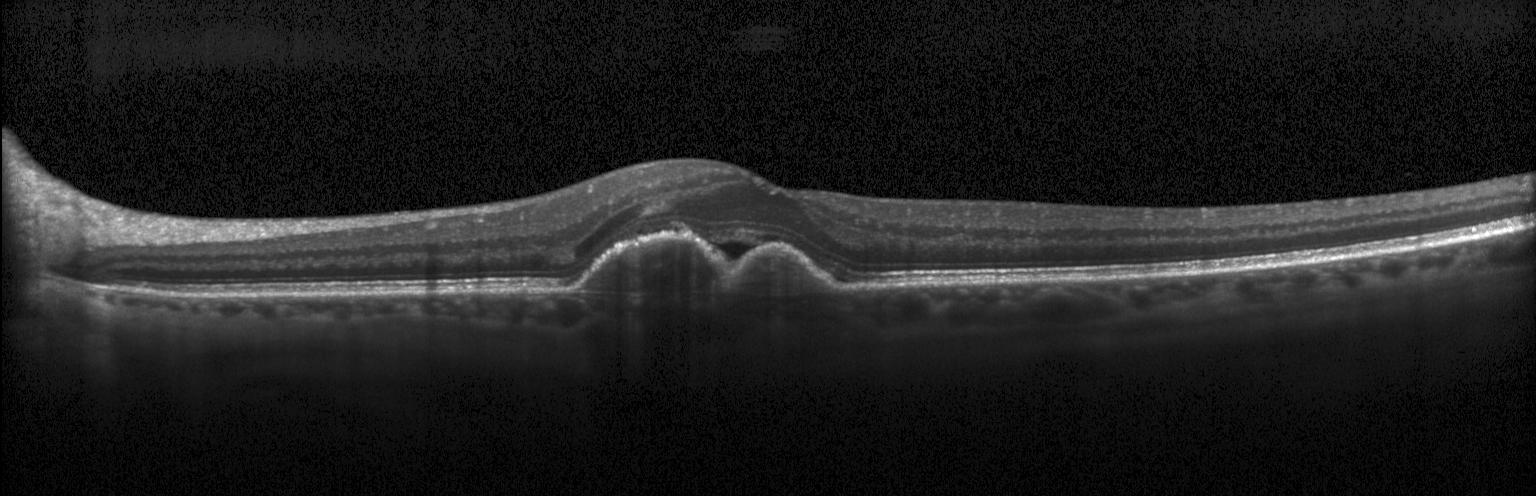
Impression: a choroidal neovascular membrane.